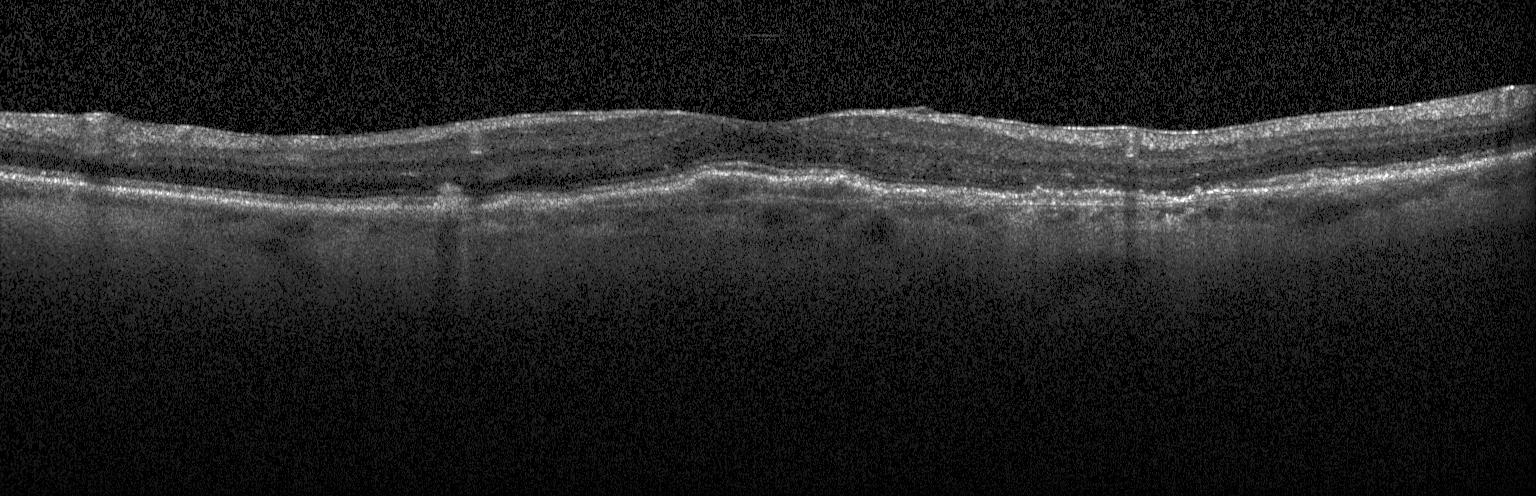
Retinal OCT cross-section showing a choroidal neovascular membrane.